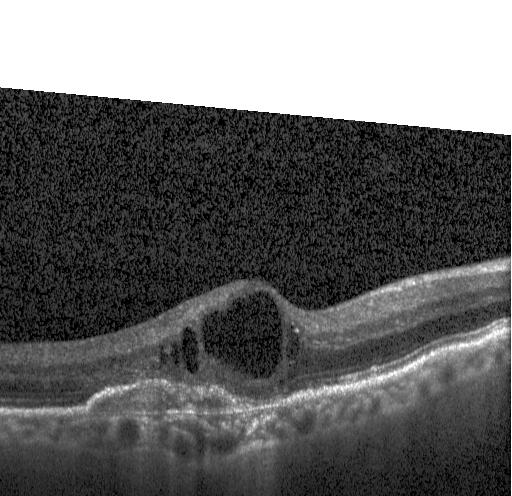

Horizontal scan through the fovea. Retinal OCT B-scan. Finding: CNV.